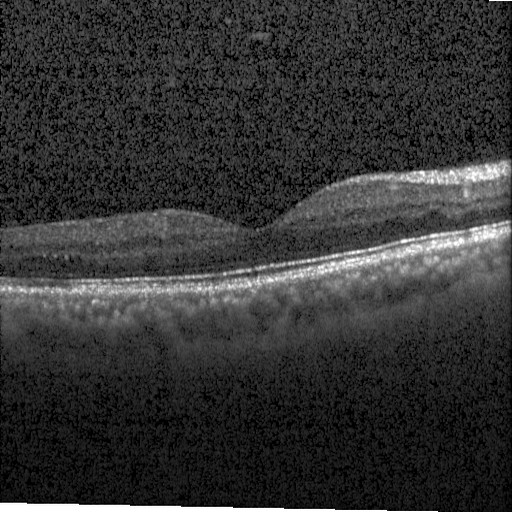
OCT line scan, spectral-domain OCT, macular scan — Finding: diabetic macular edema (DME).